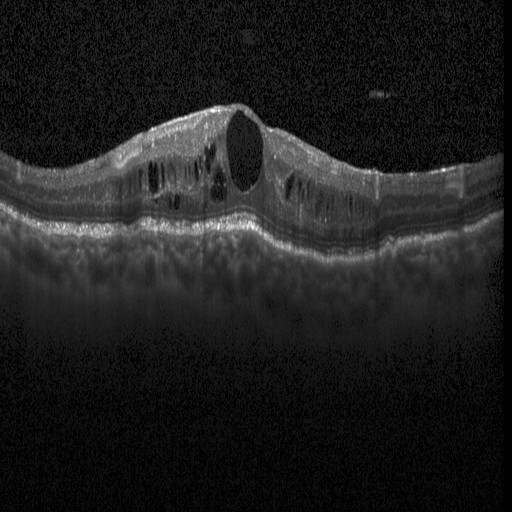
Retinal OCT B-scan. Spectral-domain OCT. Macular OCT: diabetic macular edema.